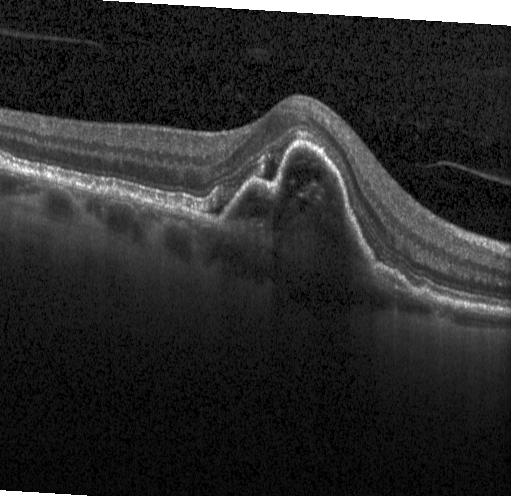 OCT B-scan.
This B-scan demonstrates a choroidal neovascular membrane.